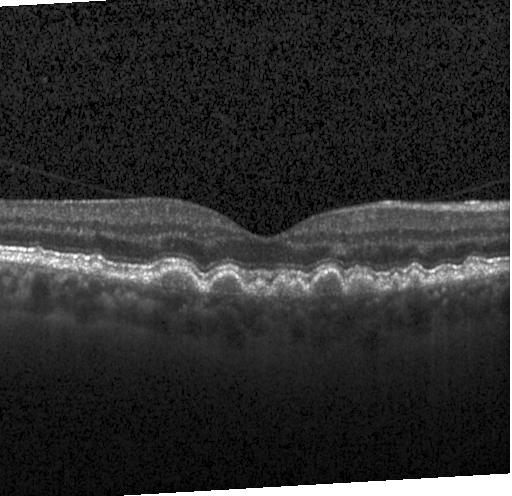 Acquired on a Heidelberg Spectralis; retinal OCT cross-section; spectral-domain OCT — The scan shows drusen.